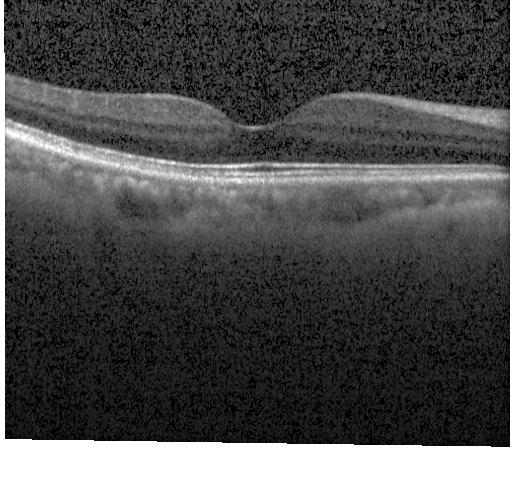

Instrument: Heidelberg Spectralis · retinal OCT B-scan — This B-scan demonstrates no CNV, no DME, and no drusen.